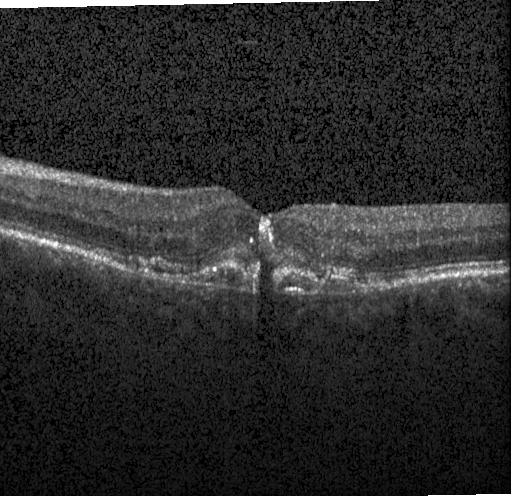

Impression: CNV.